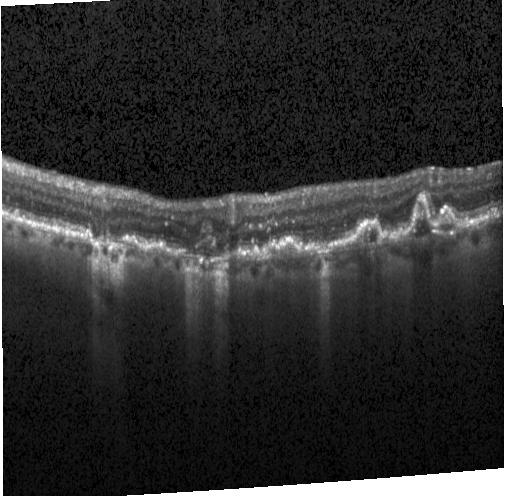

Spectral-domain OCT, Heidelberg Spectralis, centered on the fovea, retinal OCT B-scan — Finding: CNV.